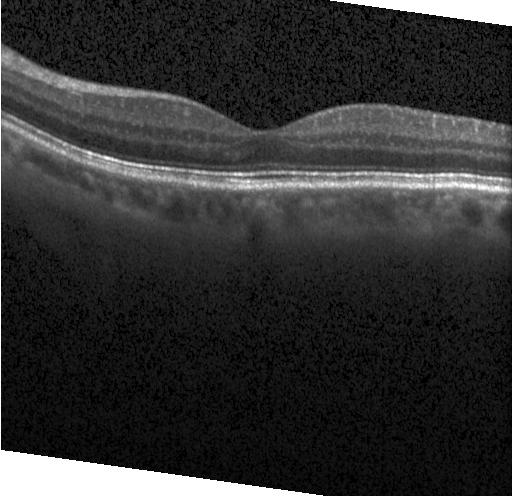
Macular scan; Heidelberg Spectralis; optical coherence tomography scan
Dx: neither choroidal neovascularization, diabetic macular edema, nor drusen.